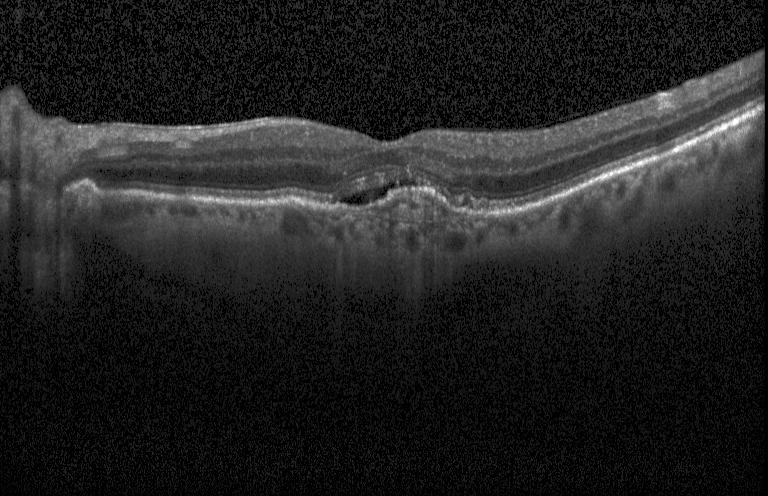 OCT scan showing a choroidal neovascular membrane.